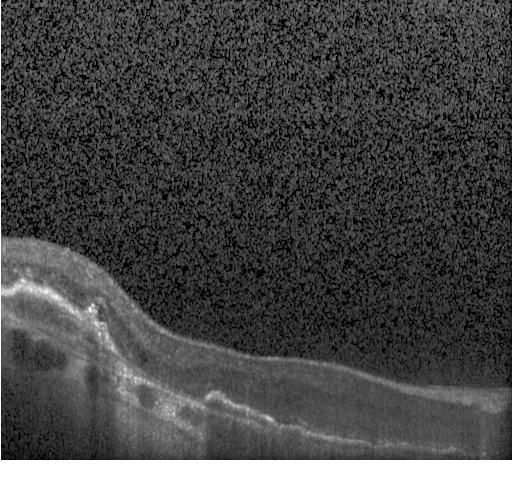
Optical coherence tomography scan; centered on the fovea; spectral-domain optical coherence tomography; Heidelberg Spectralis OCT system
Dx: a choroidal neovascular membrane.